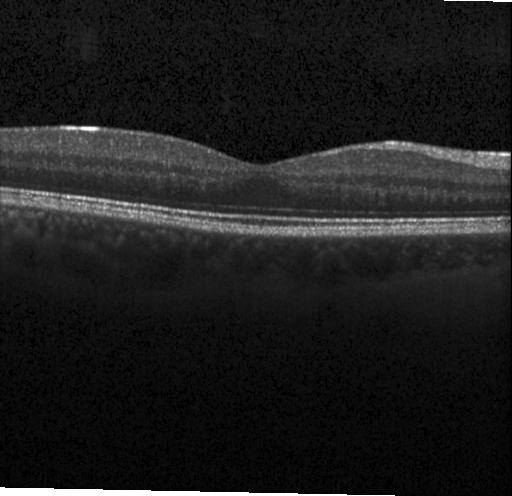

Macular OCT demonstrating neither choroidal neovascularization, diabetic macular edema, nor drusen.